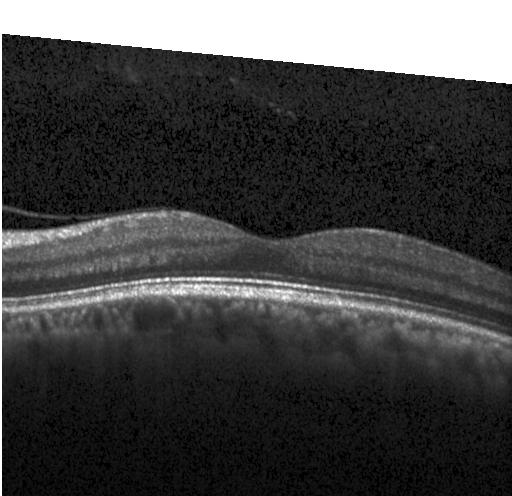

Fovea-centered. Spectral-domain optical coherence tomography. Optical coherence tomography B-scan — No choroidal neovascularization, no diabetic macular edema, and no drusen.